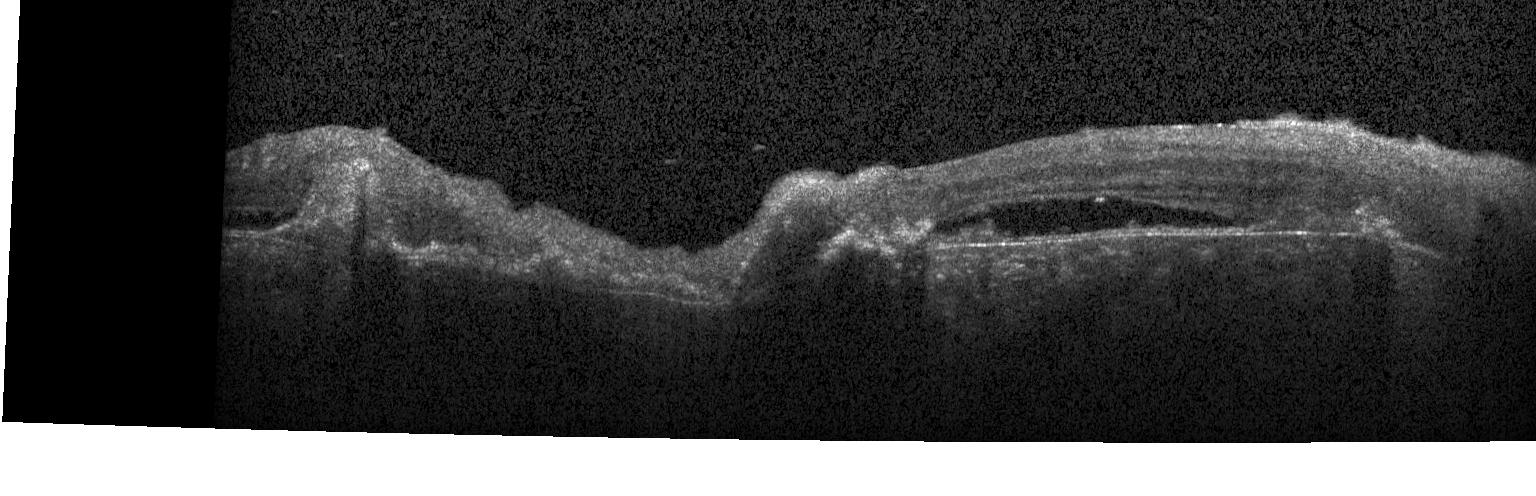
Optical coherence tomography B-scan
Macular OCT: choroidal neovascularization (CNV).